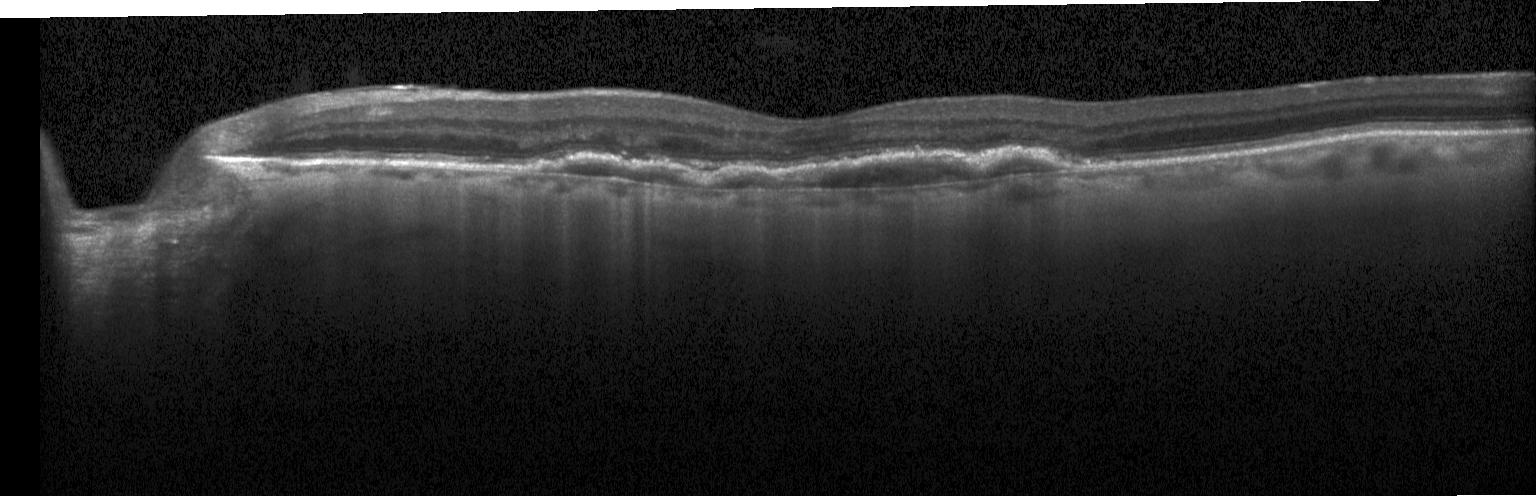
Impression: CNV.